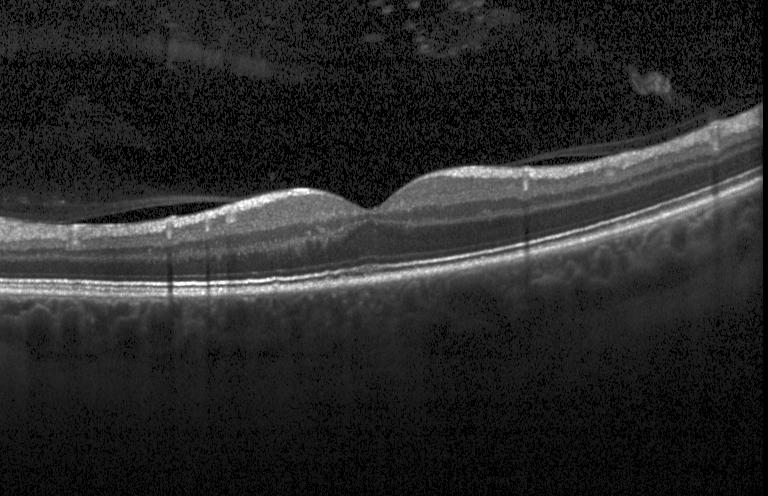
Macular OCT: no CNV, no DME, and no drusen.